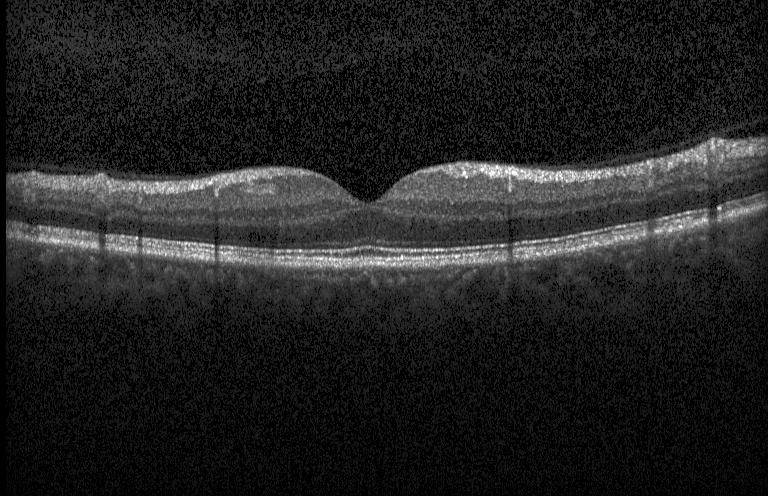 Finding: no CNV, no DME, and no drusen.